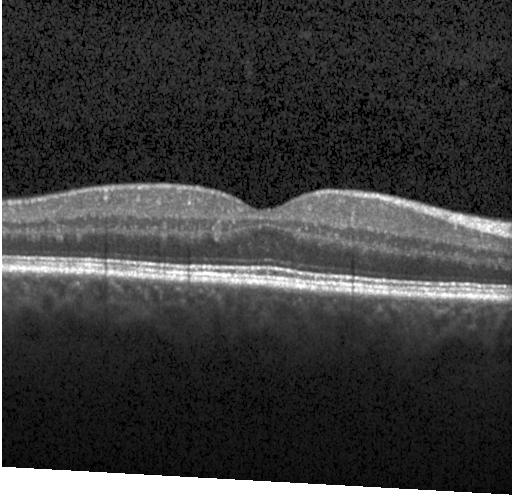

Acquired on a Heidelberg Spectralis. Macular scan. OCT line scan. Spectral-domain OCT — OCT finding: neither choroidal neovascularization, diabetic macular edema, nor drusen.